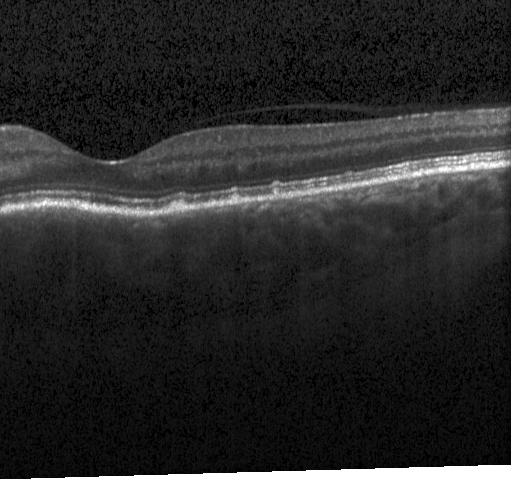 Diagnosis: sub-RPE drusenoid deposits.